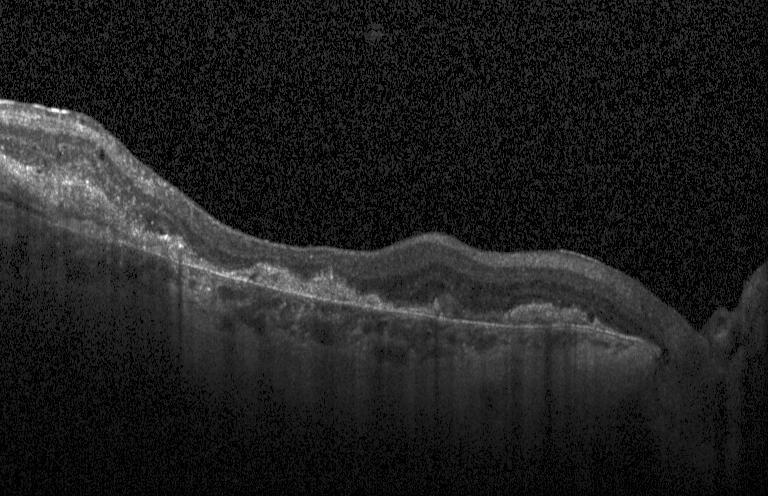 Fovea-centered, spectral-domain OCT, OCT line scan, instrument: Heidelberg Spectralis
Dx: choroidal neovascularization.